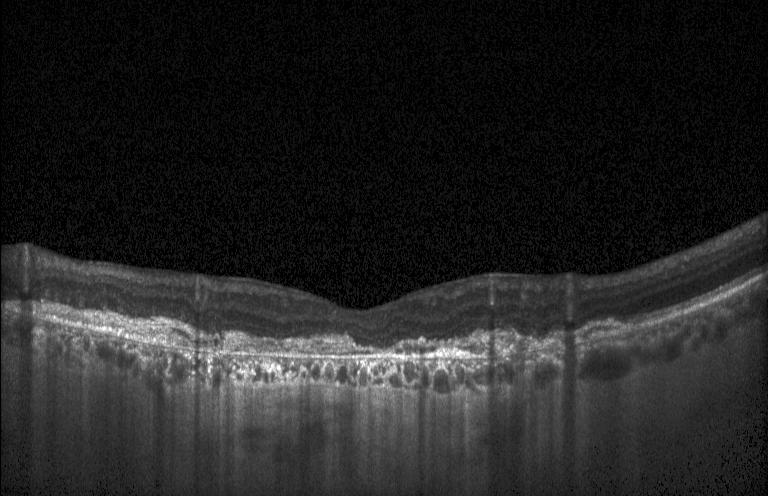

Macular OCT demonstrating a choroidal neovascular membrane.